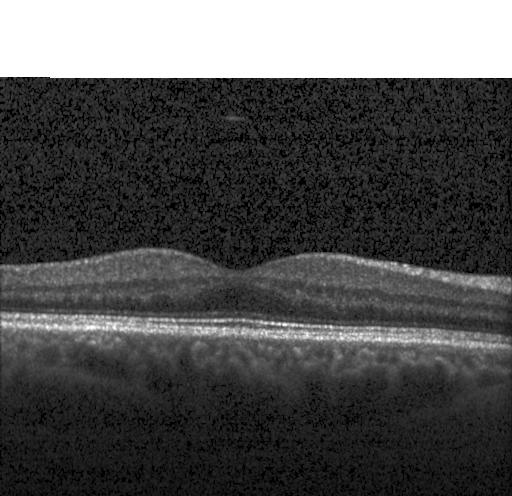

Diagnosis: no evidence of choroidal neovascularization, diabetic macular edema, or drusen.